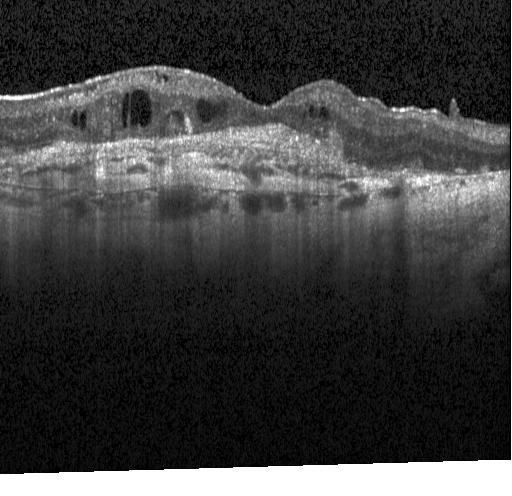 OCT scan showing choroidal neovascularization.